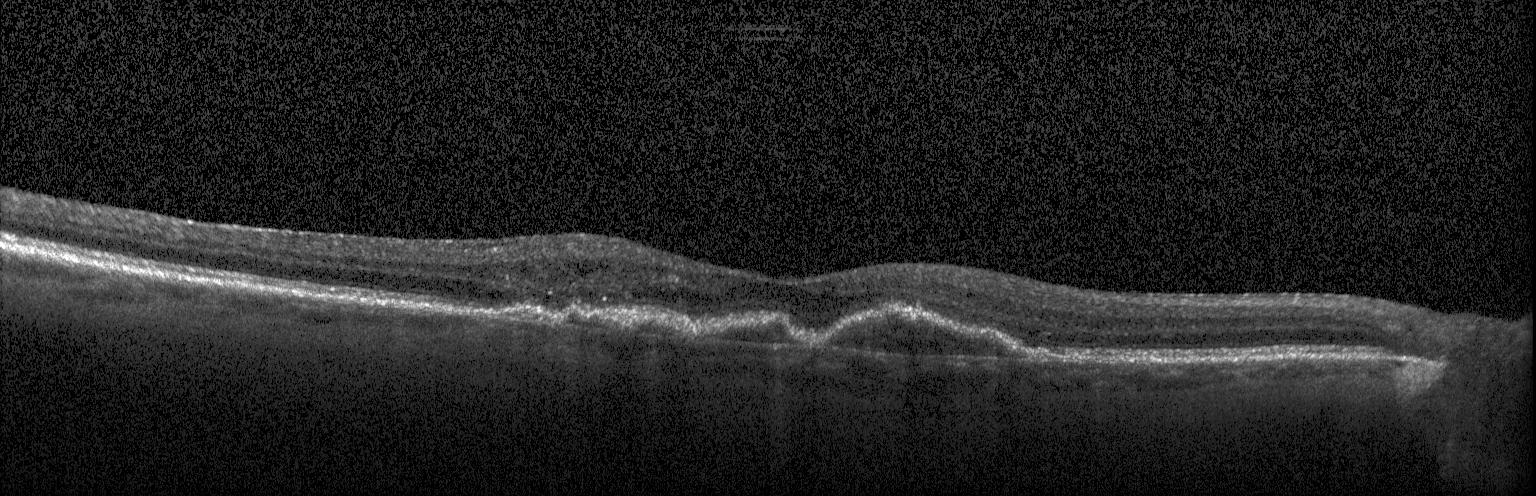

OCT B-scan, horizontal scan through the fovea. Macular OCT: a choroidal neovascular membrane.